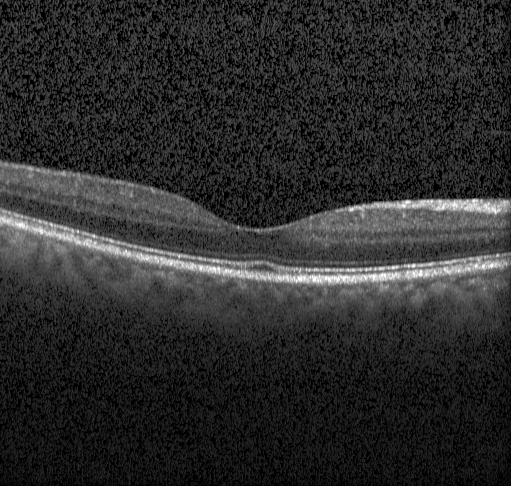 Acquired on a Heidelberg Spectralis, macular scan, OCT line scan.
The scan shows no CNV, no DME, and no drusen.